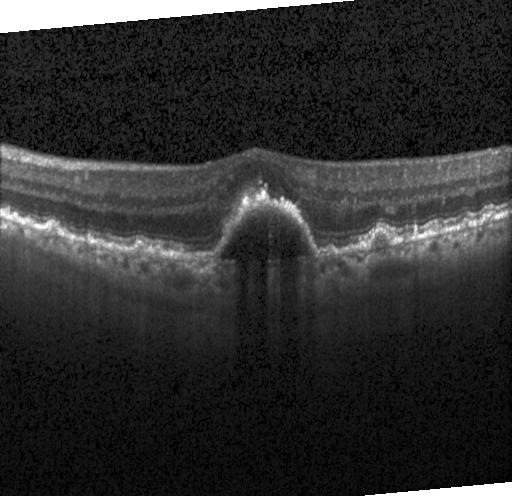

Optical coherence tomography scan. Horizontal scan through the fovea. SD-OCT — Impression: choroidal neovascularization.